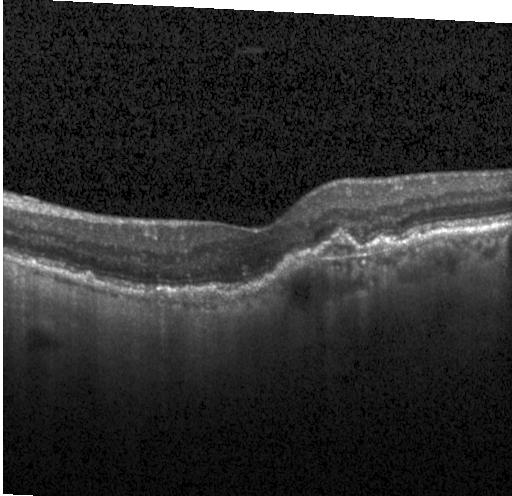 OCT line scan. The scan shows a choroidal neovascular membrane.